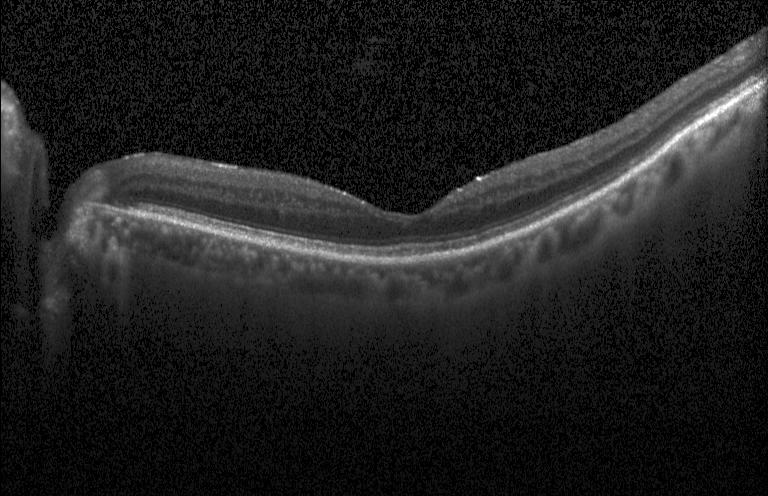 Retinal OCT cross-section · spectral-domain OCT — Diagnosis: no evidence of CNV, DME, or drusen.